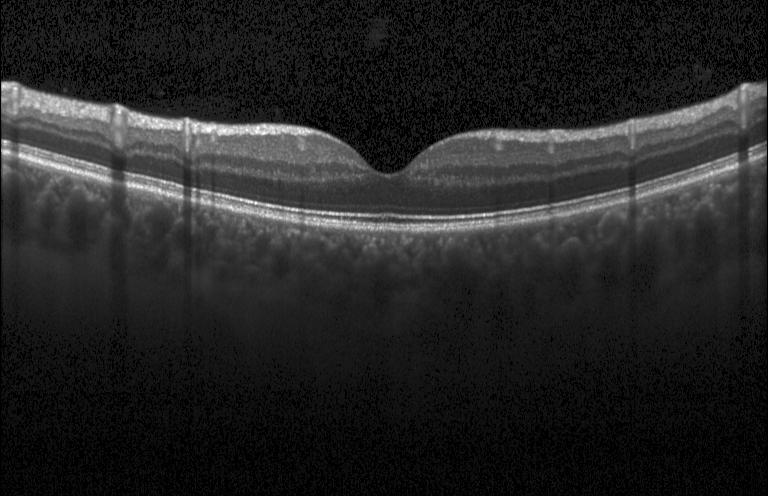

Spectral-domain OCT B-scan: neither CNV, DME, nor drusen.